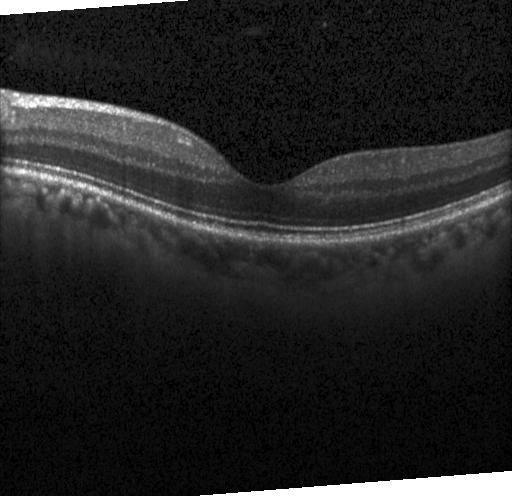 Macular scan · instrument: Heidelberg Spectralis · retinal OCT cross-section
Neither choroidal neovascularization, diabetic macular edema, nor drusen.